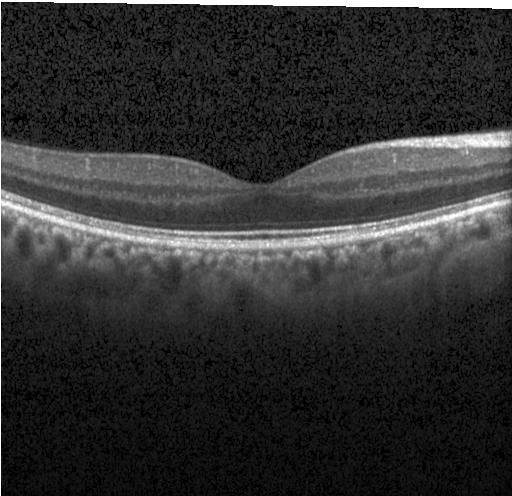

Dx: neither choroidal neovascularization, diabetic macular edema, nor drusen.